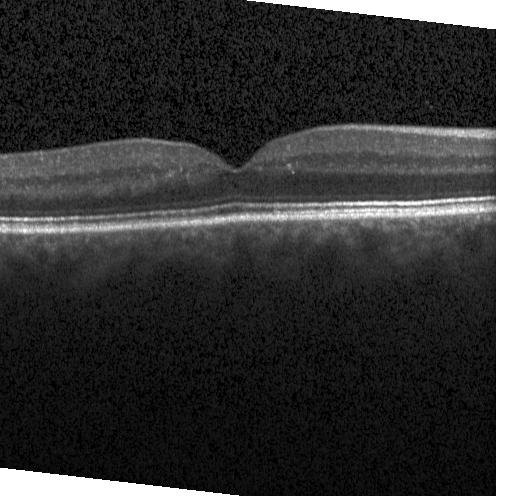 Macular OCT: no evidence of choroidal neovascularization, diabetic macular edema, or drusen.